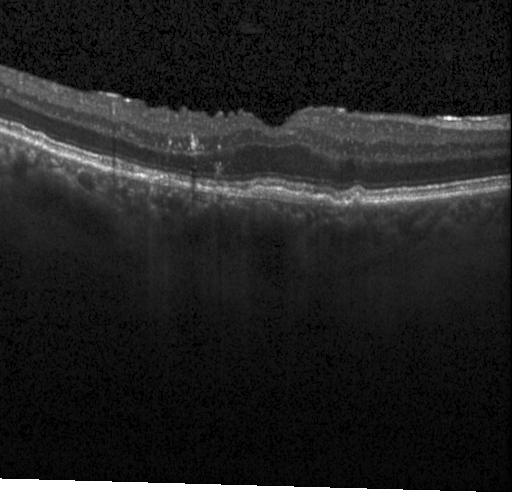
Retinal OCT cross-section.
This B-scan demonstrates a choroidal neovascular membrane.